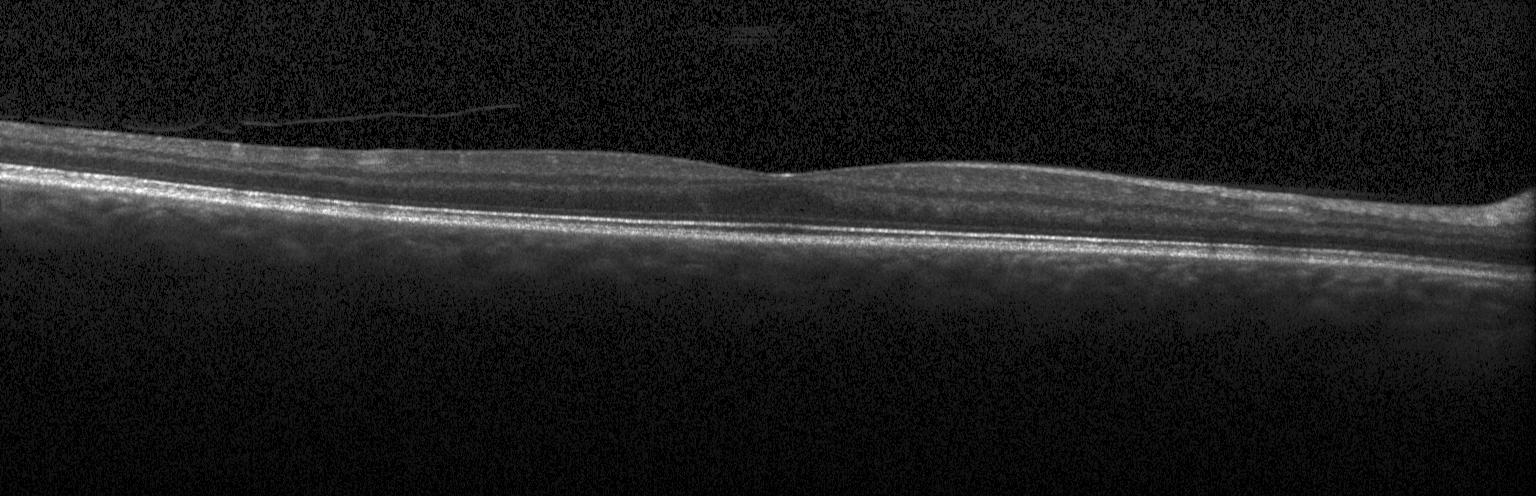 Heidelberg Spectralis OCT system; retinal OCT cross-section; spectral-domain optical coherence tomography; through the macula — Dx: no CNV, DME, or drusen.